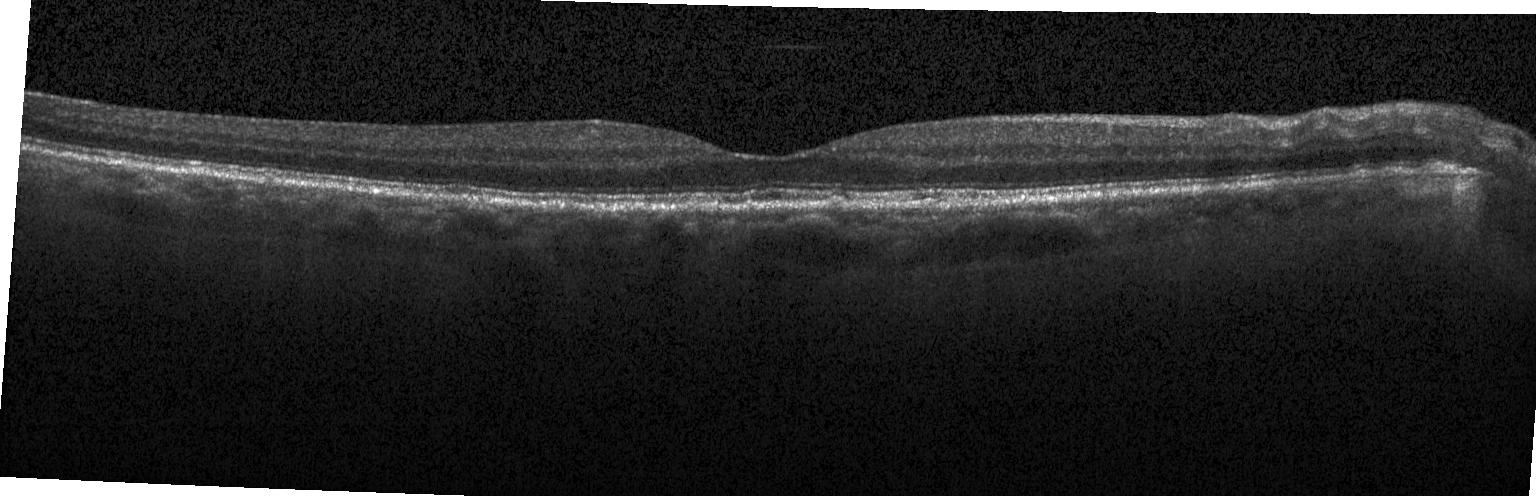
Optical coherence tomography scan, horizontal scan through the fovea, Heidelberg Spectralis — Multiple drusen.